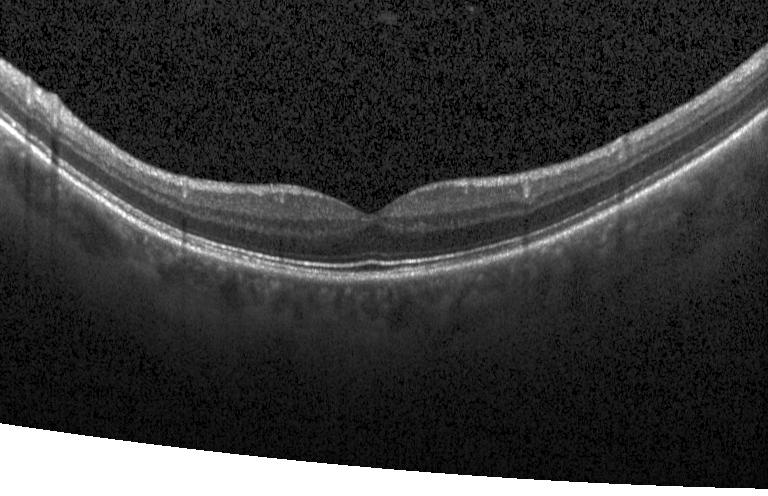

Spectral-domain OCT B-scan: no choroidal neovascularization, diabetic macular edema, or drusen.